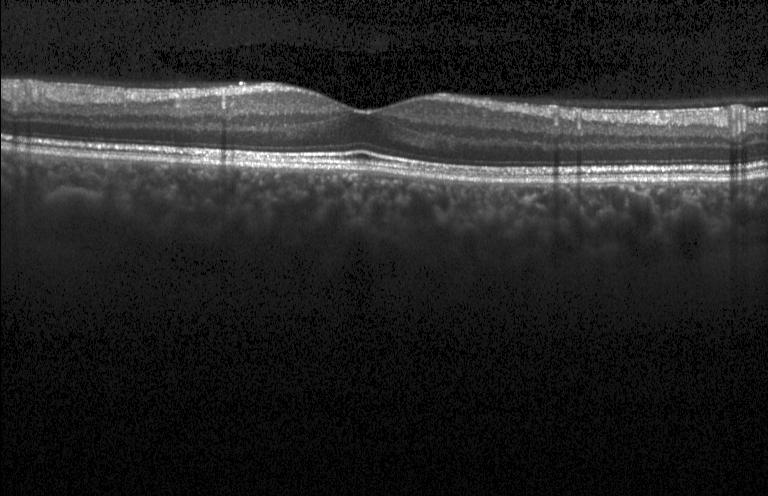
Optical coherence tomography B-scan — Impression: no CNV, DME, or drusen.